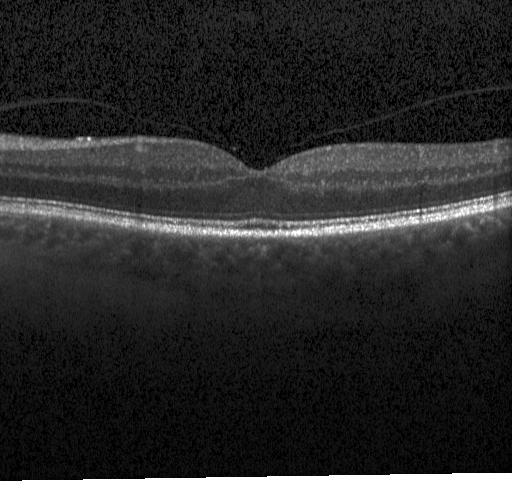 Retinal OCT B-scan
This B-scan demonstrates no CNV, no DME, and no drusen.